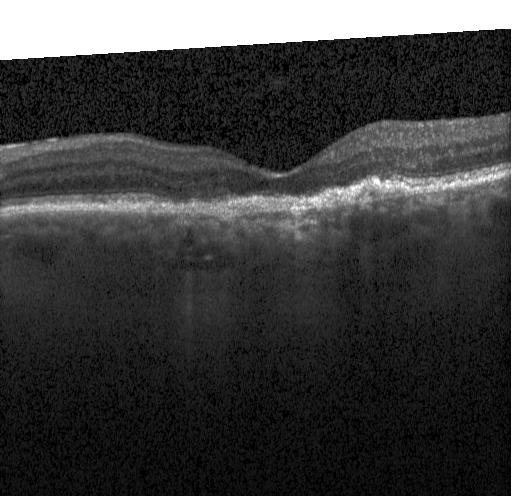
Retinal OCT cross-section — The scan shows choroidal neovascularization (CNV).